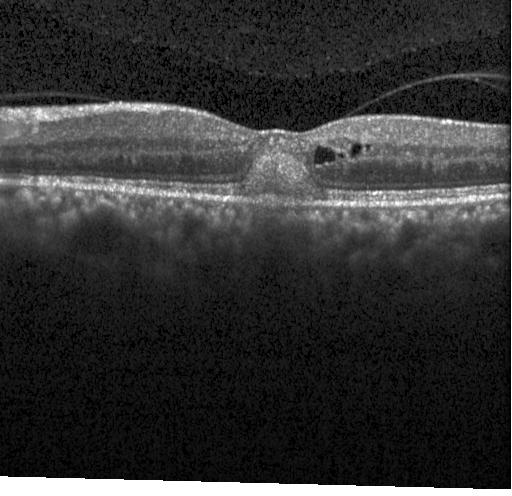 Finding: CNV.